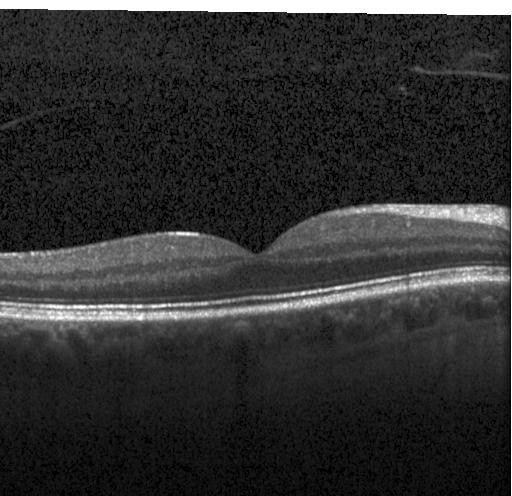 OCT line scan. Spectral-domain optical coherence tomography. Instrument: Heidelberg Spectralis — The scan shows no CNV, DME, or drusen.